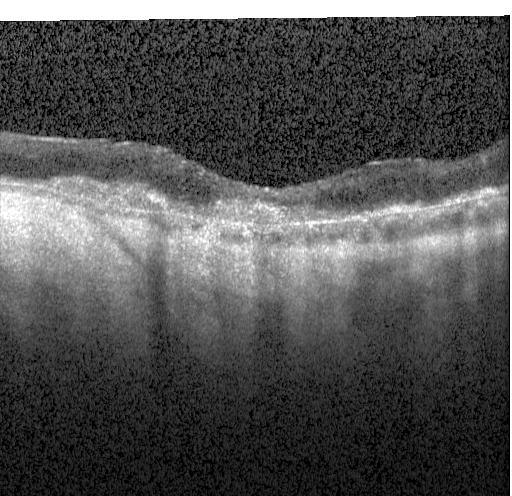
Assessment: CNV.